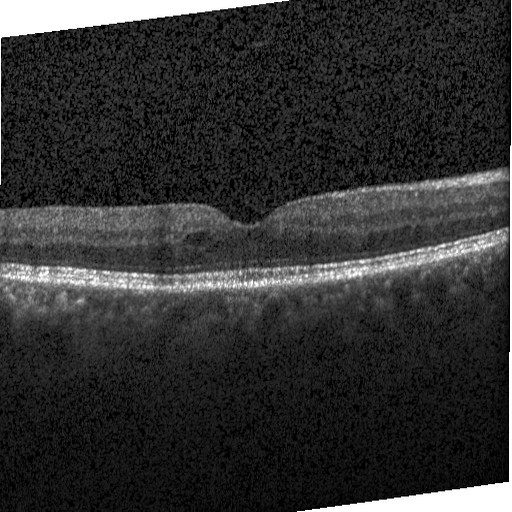 Retinal OCT cross-section; horizontal scan through the fovea.
Dx: diabetic macular edema (DME).